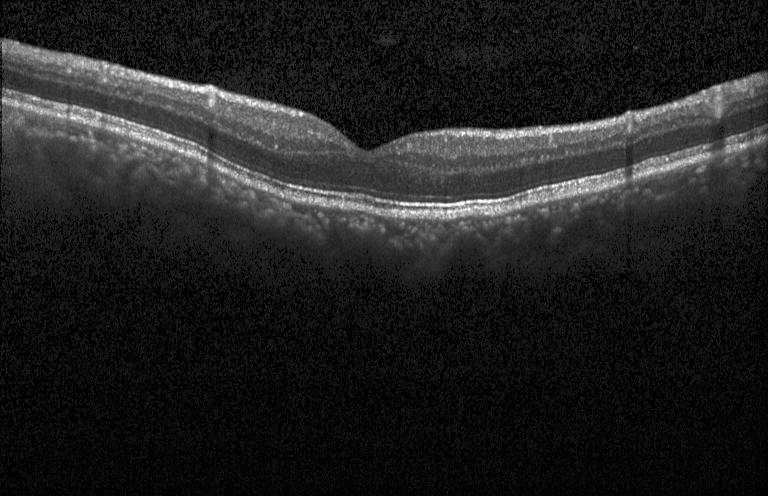
Finding: no CNV, DME, or drusen.